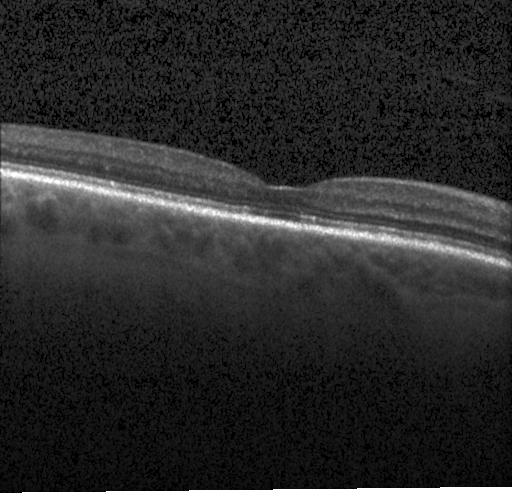 Optical coherence tomography scan. Spectral-domain optical coherence tomography — Diagnosis: no choroidal neovascularization, diabetic macular edema, or drusen.